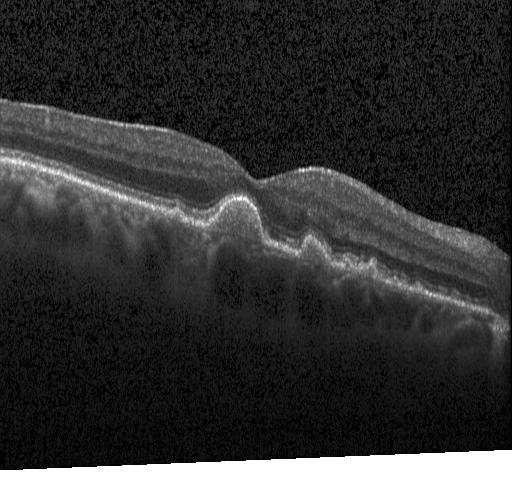 Spectral-domain OCT · optical coherence tomography scan · instrument: Heidelberg Spectralis · horizontal scan through the fovea — Assessment: multiple drusen.